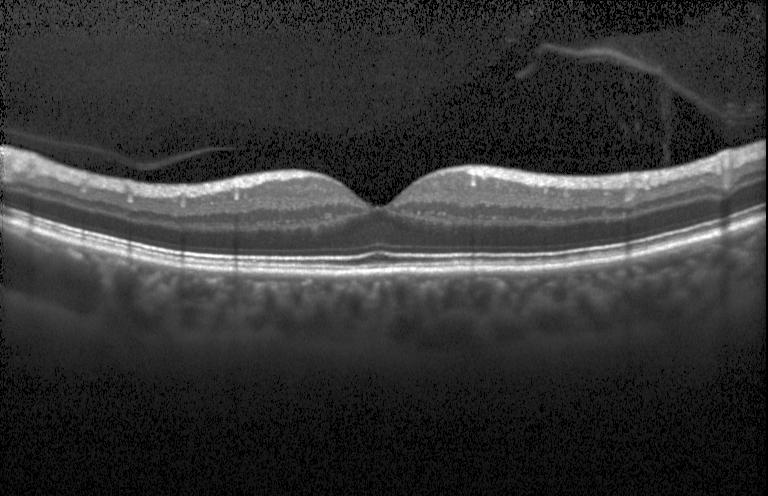

Heidelberg Spectralis · SD-OCT · optical coherence tomography B-scan · fovea-centered
Finding: no CNV, no DME, and no drusen.